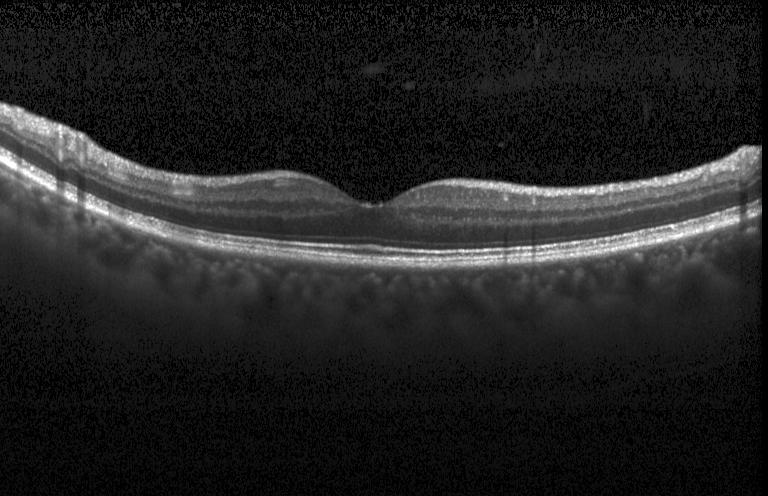 OCT finding: no evidence of CNV, DME, or drusen.